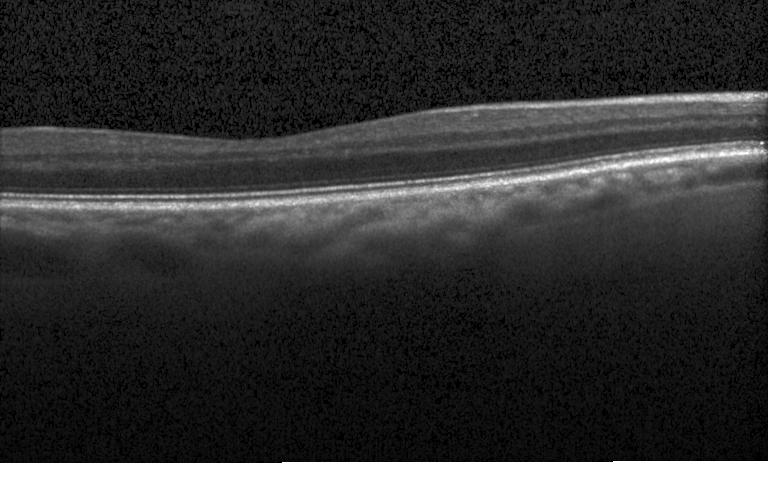 Fovea-centered · spectral-domain optical coherence tomography · OCT line scan — Dx: no evidence of choroidal neovascularization, diabetic macular edema, or drusen.